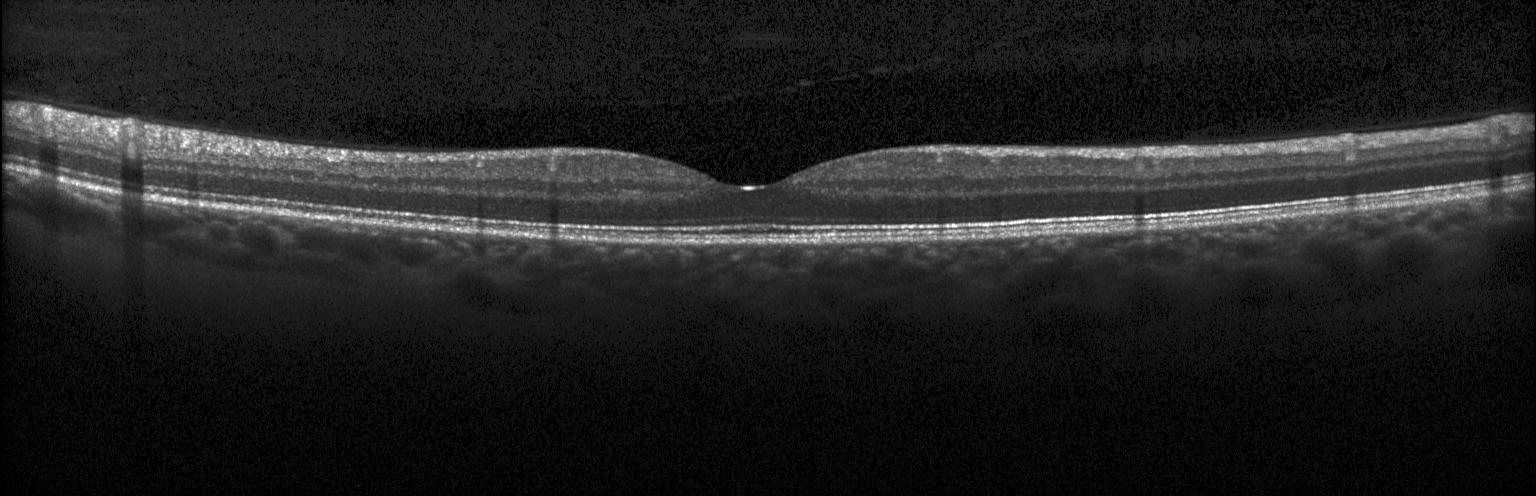

OCT B-scan — The scan shows neither CNV, DME, nor drusen.